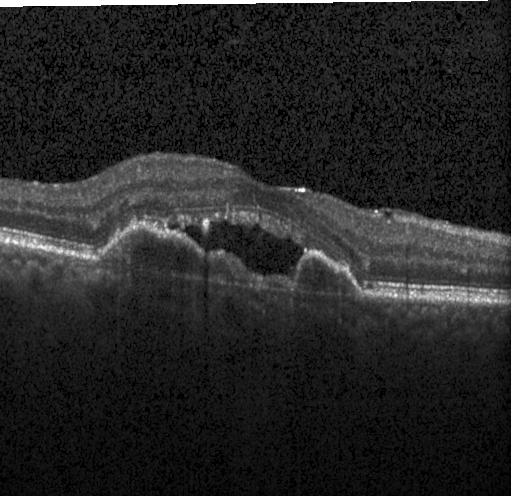
Macular OCT: choroidal neovascularization.